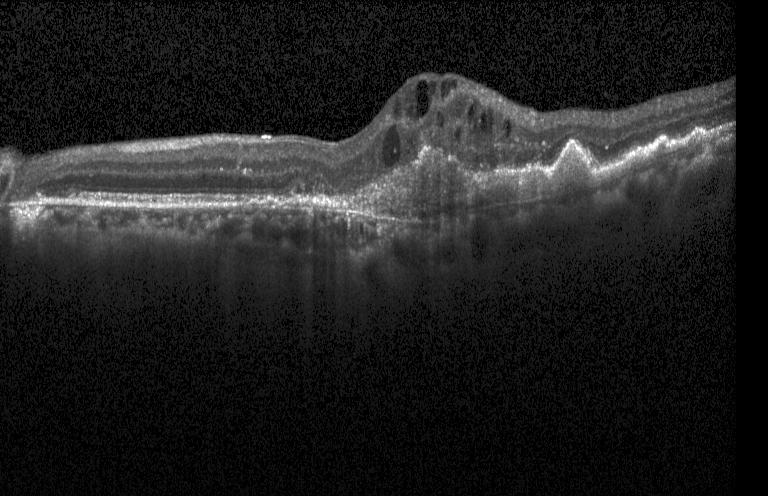 Diagnosis: choroidal neovascularization (CNV).